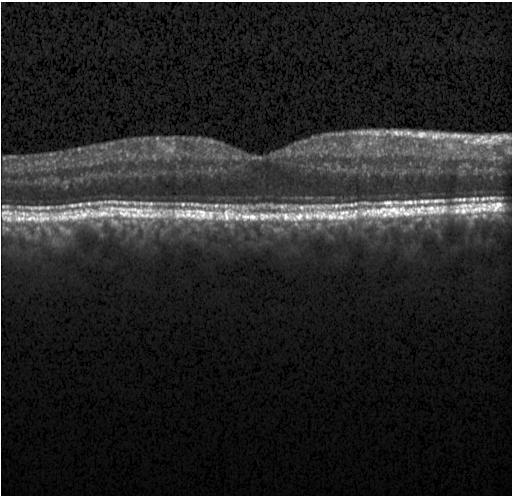 Optical coherence tomography B-scan. Fovea-centered — Finding: neither choroidal neovascularization, diabetic macular edema, nor drusen.